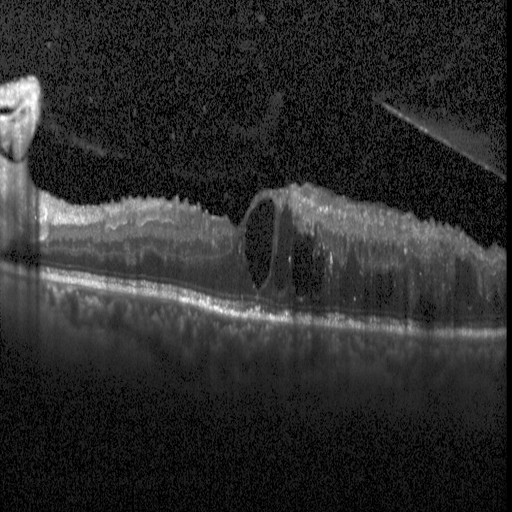

OCT B-scan · spectral-domain OCT · macular scan · instrument: Heidelberg Spectralis
The scan shows DME.